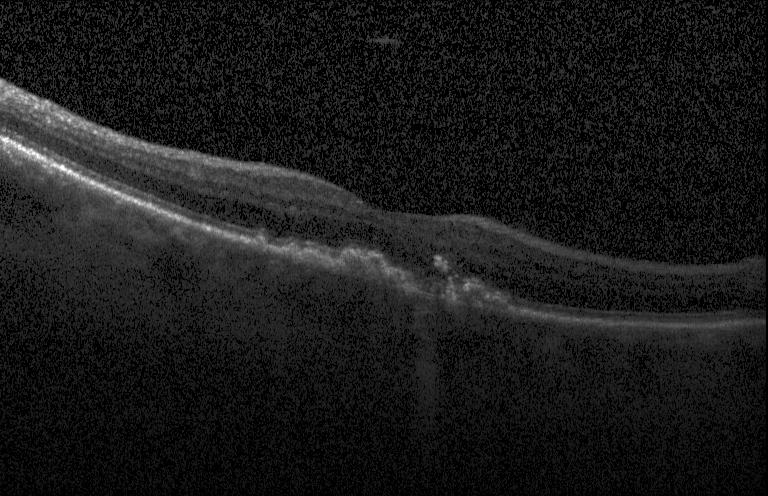

Assessment: CNV.